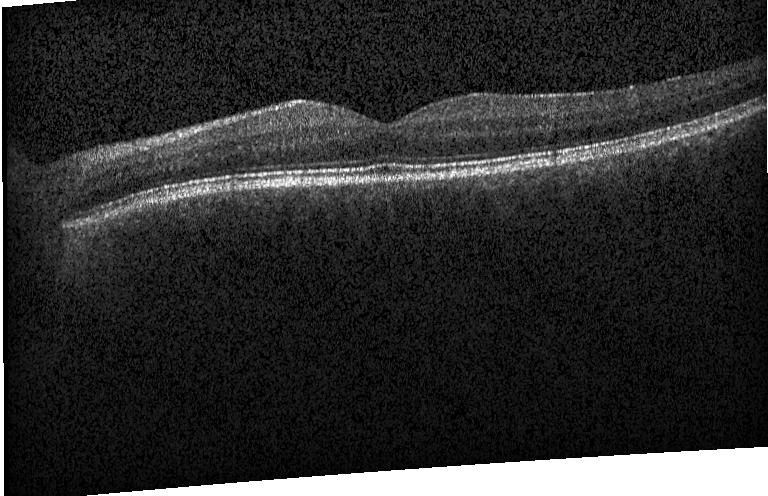

SD-OCT, OCT line scan.
Neither choroidal neovascularization, diabetic macular edema, nor drusen.